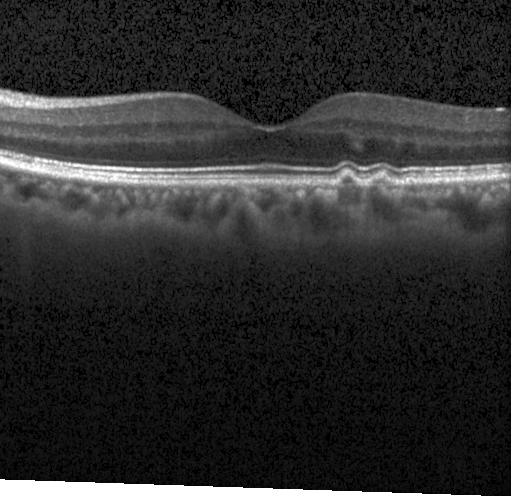
Retinal OCT cross-section showing drusen.